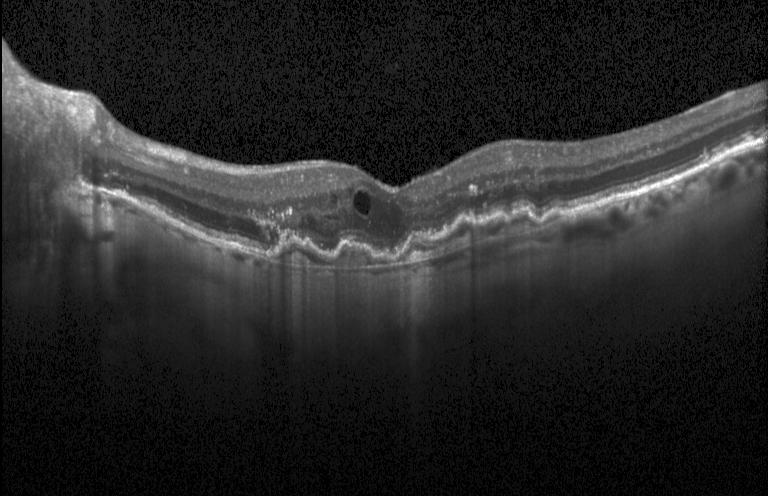 Diagnosis: CNV.